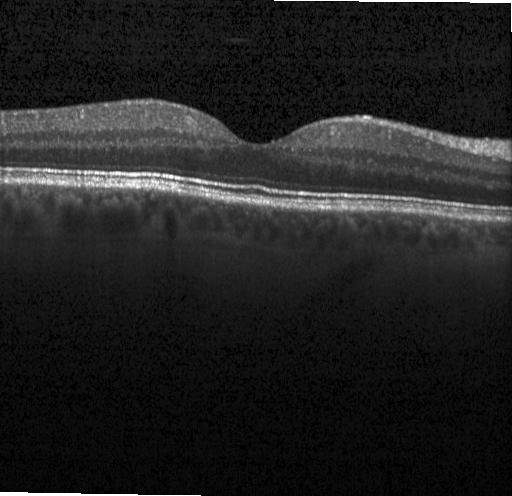 Fovea-centered. Heidelberg Spectralis. Spectral-domain optical coherence tomography. Optical coherence tomography B-scan — Dx: no evidence of choroidal neovascularization, diabetic macular edema, or drusen.